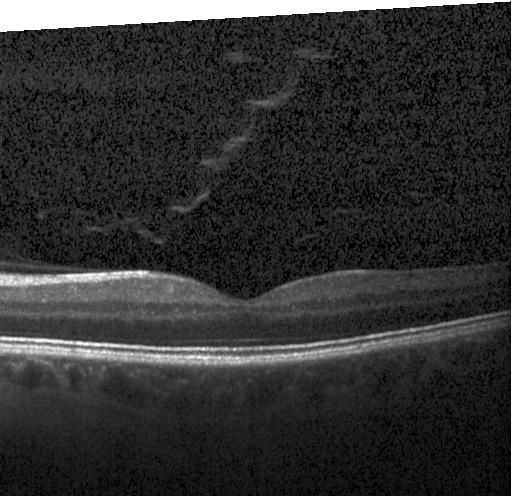 Dx: no evidence of choroidal neovascularization, diabetic macular edema, or drusen.